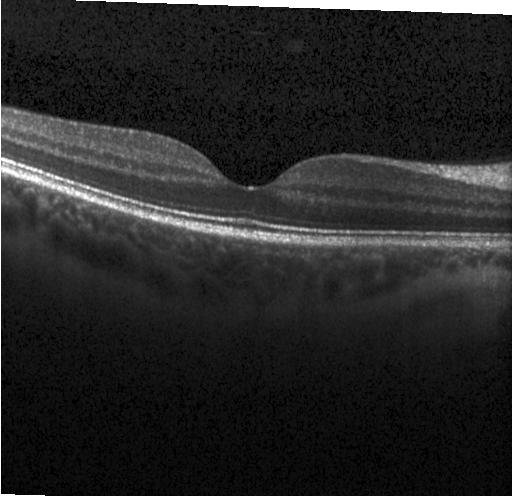

Spectral-domain OCT, Heidelberg Spectralis, centered on the fovea, optical coherence tomography scan. Diagnosis: no choroidal neovascularization, diabetic macular edema, or drusen.